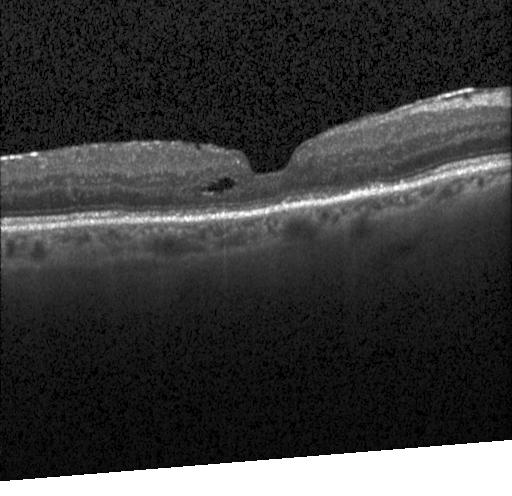

Optical coherence tomography B-scan.
This B-scan demonstrates DME.